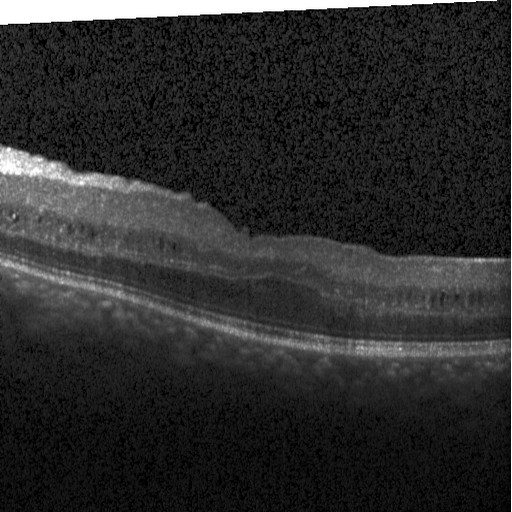
OCT scan showing DME.